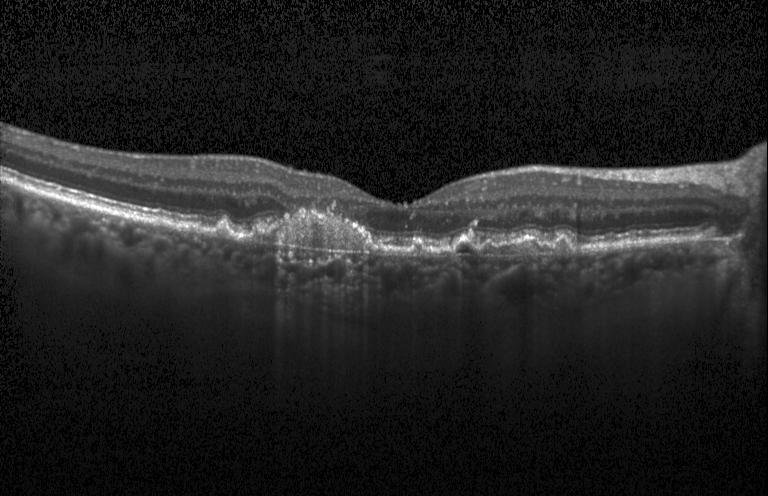 Impression: a choroidal neovascular membrane.